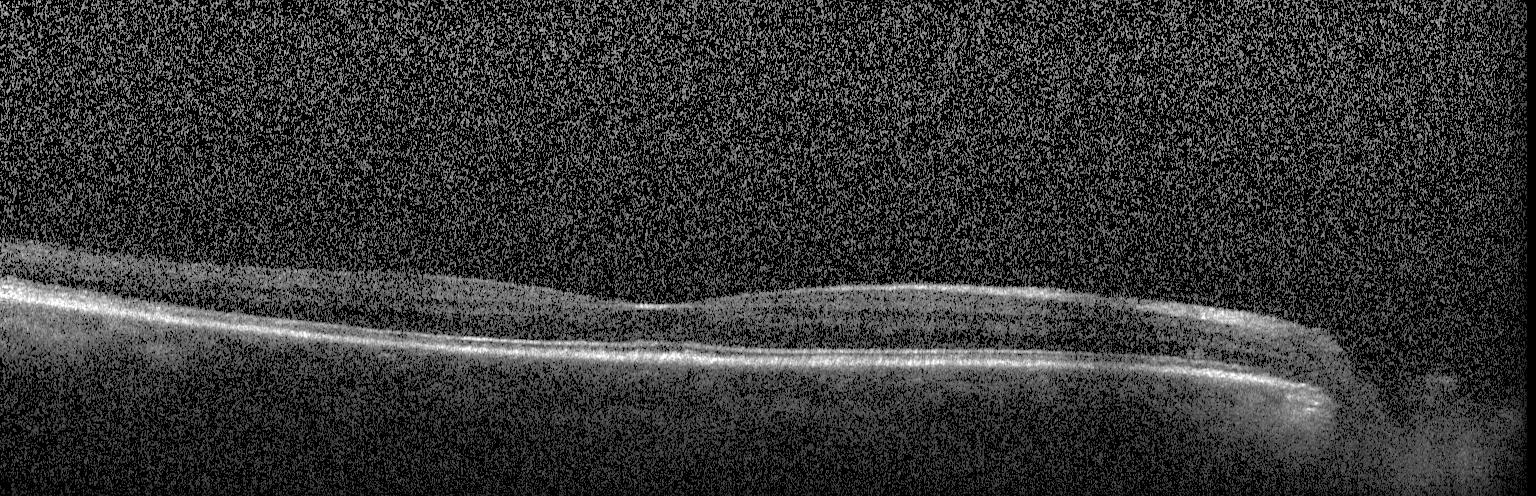

Retinal OCT cross-section showing neither CNV, DME, nor drusen.